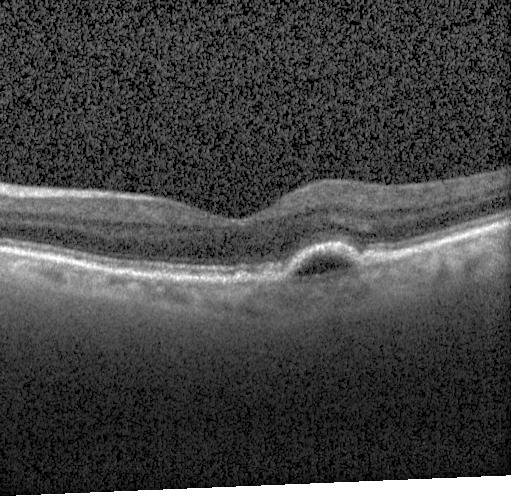

Retinal OCT B-scan
Impression: choroidal neovascularization.